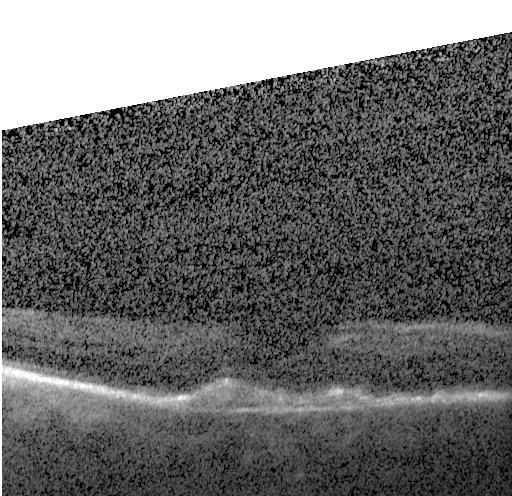 Spectral-domain optical coherence tomography, optical coherence tomography B-scan
The scan shows choroidal neovascularization (CNV).